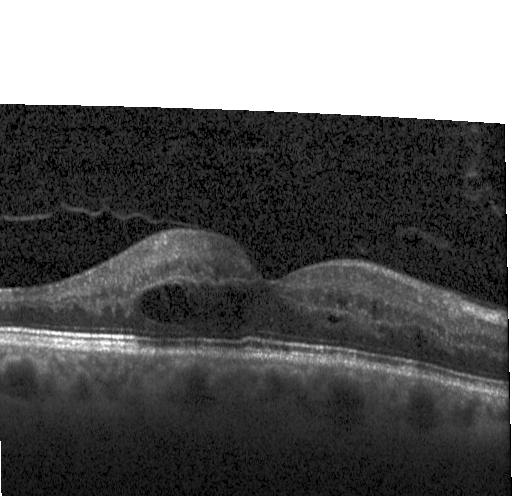

Macular OCT demonstrating diabetic macular edema (DME).